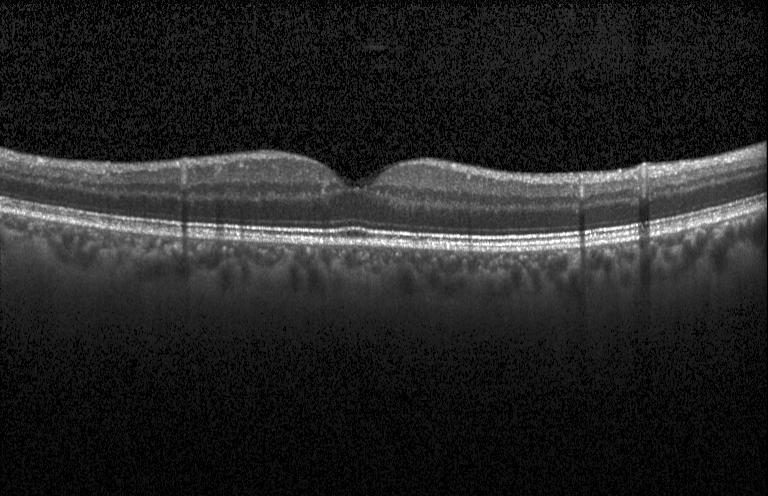
Optical coherence tomography B-scan — Diagnosis: neither choroidal neovascularization, diabetic macular edema, nor drusen.